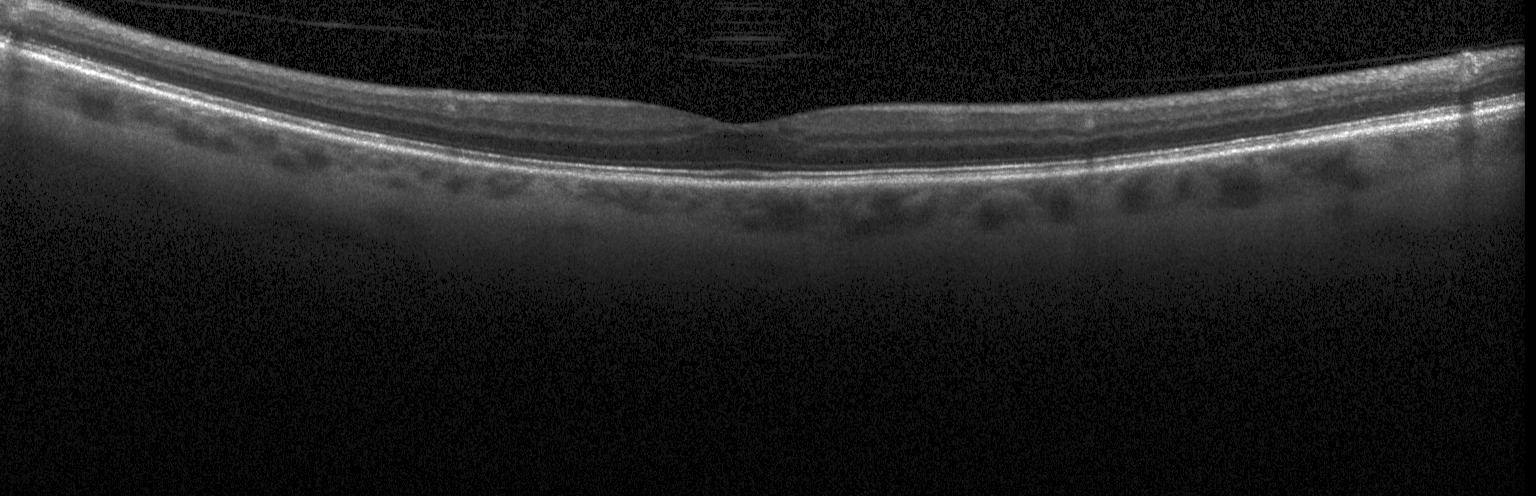

Macular OCT demonstrating neither choroidal neovascularization, diabetic macular edema, nor drusen.